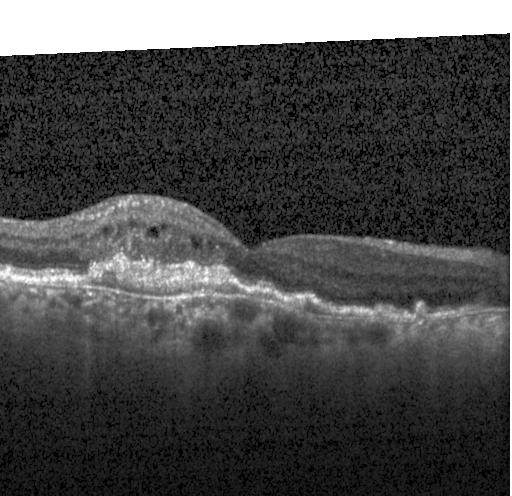
OCT B-scan showing CNV.